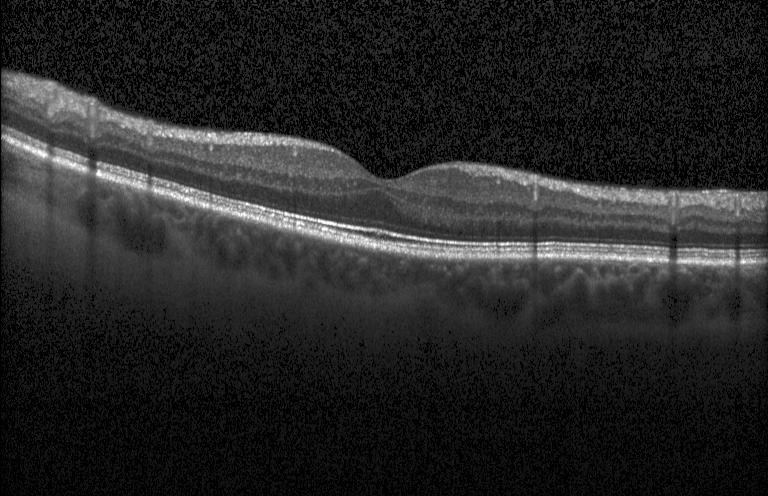

Spectral-domain optical coherence tomography, OCT line scan, through the macula, Heidelberg Spectralis OCT system. Macular OCT: no CNV, no DME, and no drusen.